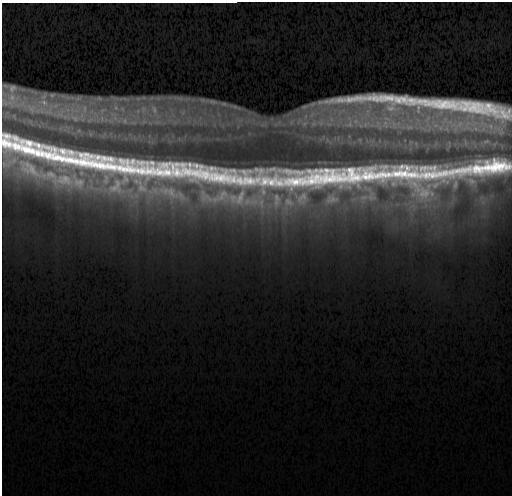

No evidence of CNV, DME, or drusen.